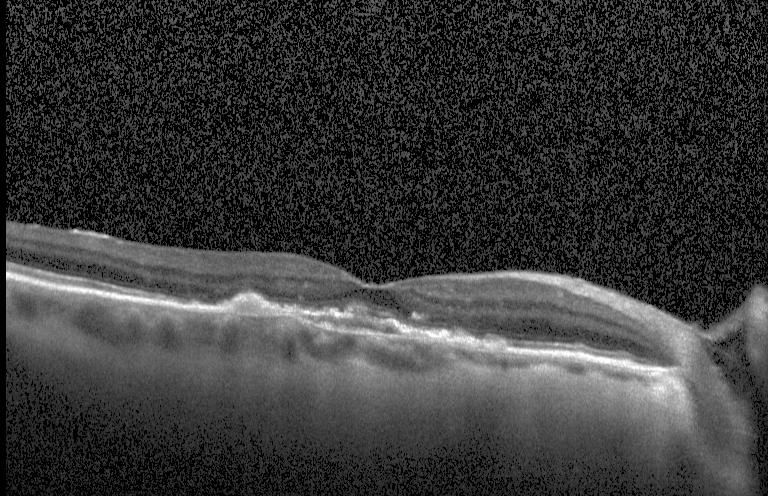 Spectral-domain OCT · OCT line scan · instrument: Heidelberg Spectralis · fovea-centered
Assessment: a choroidal neovascular membrane.